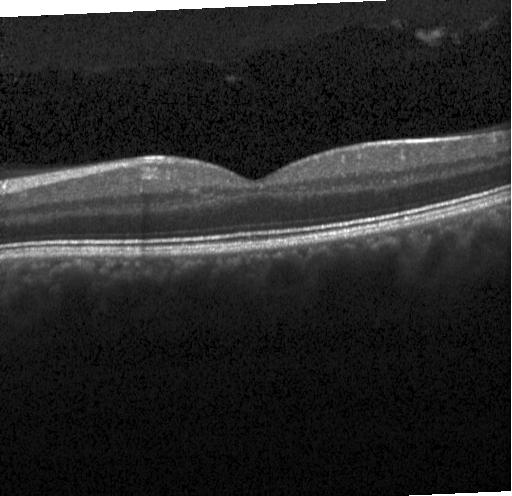 Spectral-domain OCT B-scan: no choroidal neovascularization, no diabetic macular edema, and no drusen.